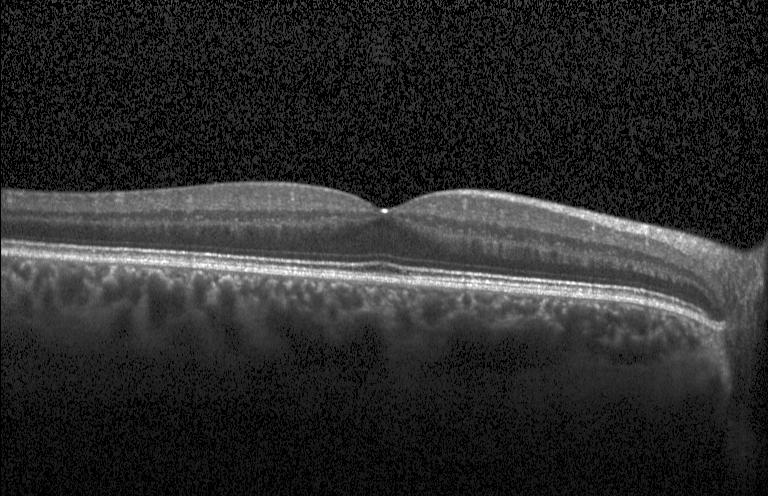 Macular OCT: no evidence of choroidal neovascularization, diabetic macular edema, or drusen.